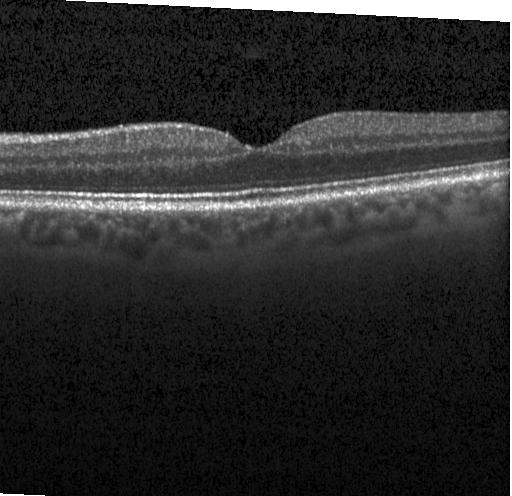 Optical coherence tomography scan · spectral-domain OCT · instrument: Heidelberg Spectralis · through the macula.
No choroidal neovascularization, no diabetic macular edema, and no drusen.